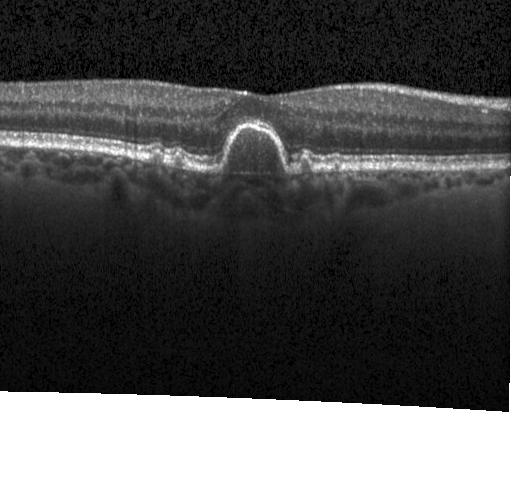

Spectral-domain OCT B-scan: a choroidal neovascular membrane.